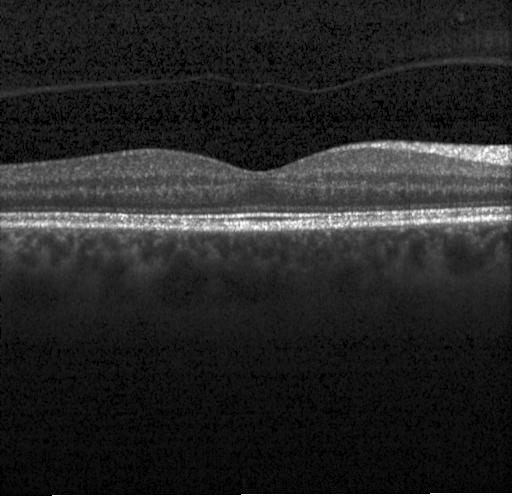
Diagnosis: no CNV, DME, or drusen.